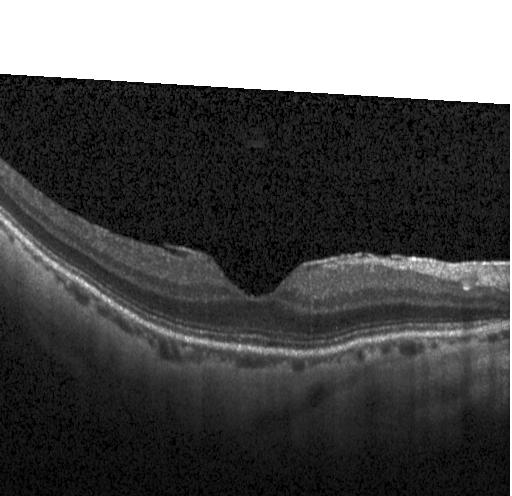
Macular OCT: neither choroidal neovascularization, diabetic macular edema, nor drusen.